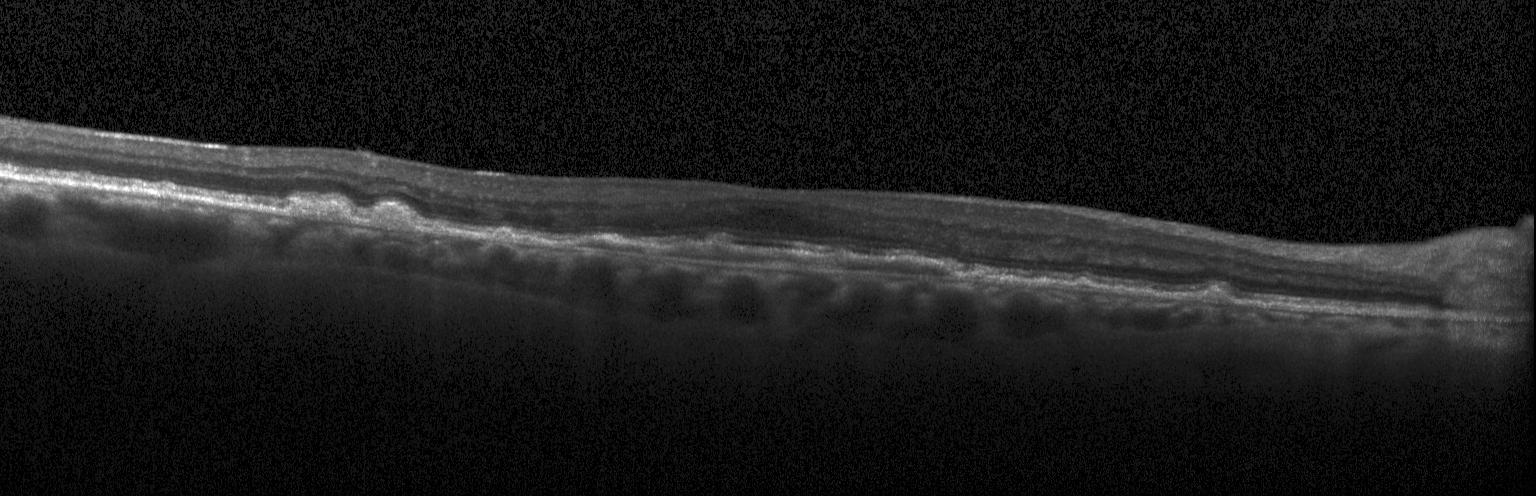 This B-scan demonstrates a choroidal neovascular membrane.